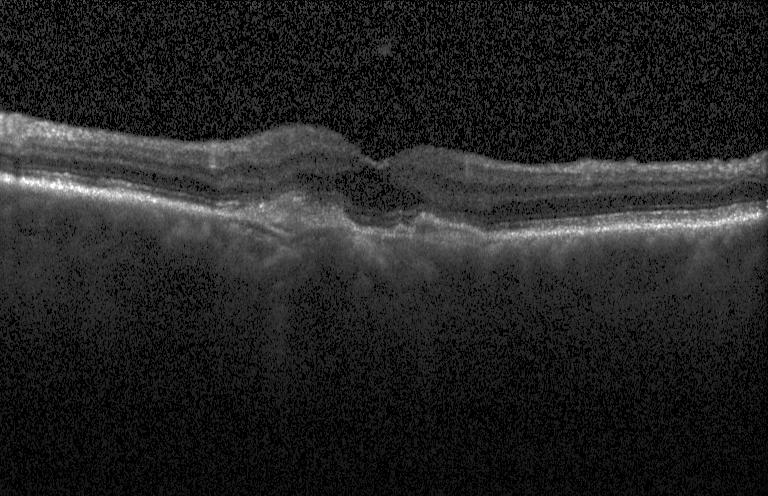

Macular OCT: CNV.